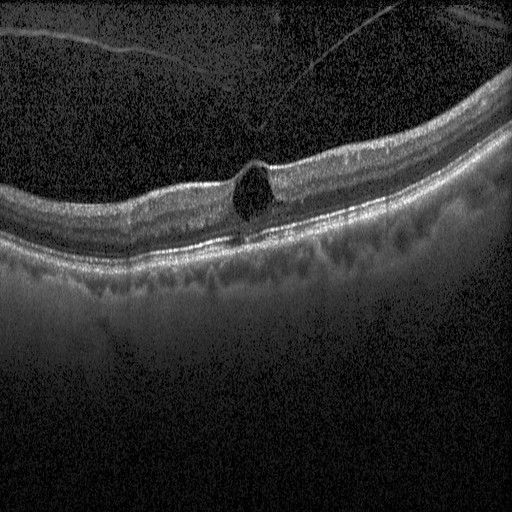 Macular scan; instrument: Heidelberg Spectralis; retinal OCT B-scan; SD-OCT
DME.